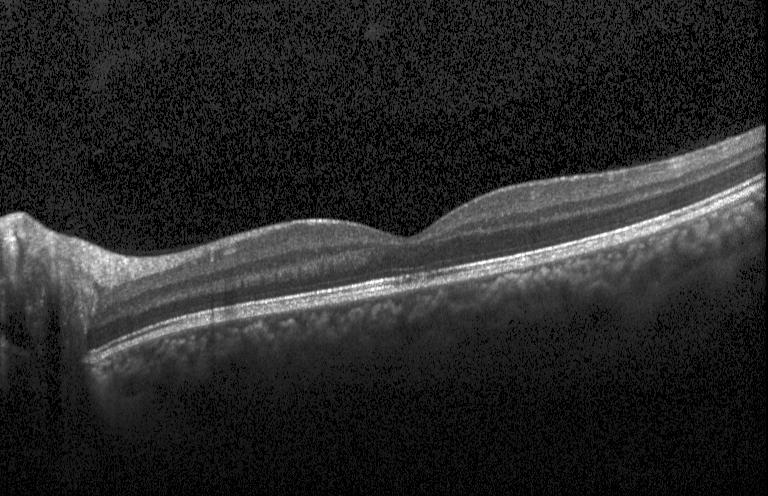
Retinal OCT cross-section showing no choroidal neovascularization, diabetic macular edema, or drusen.